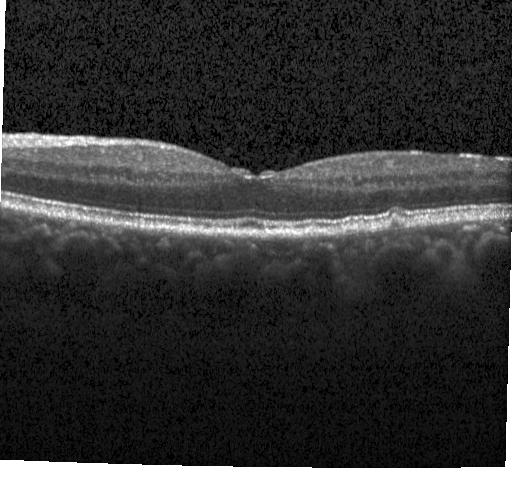

The scan shows drusen.